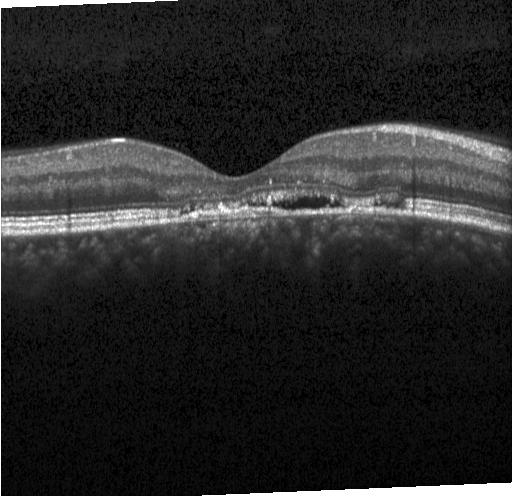 Optical coherence tomography B-scan
Diagnosis: a choroidal neovascular membrane.